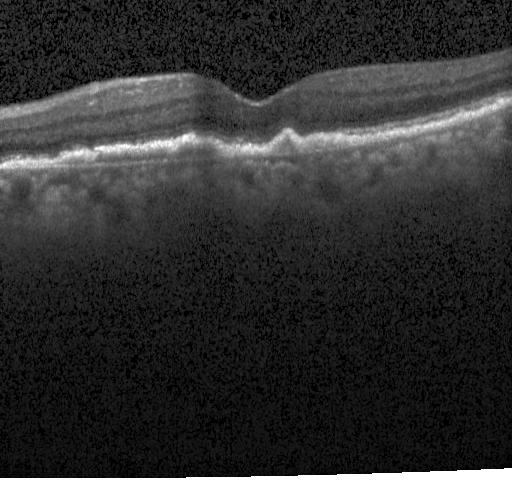
OCT B-scan; Heidelberg Spectralis OCT system. Impression: a choroidal neovascular membrane.